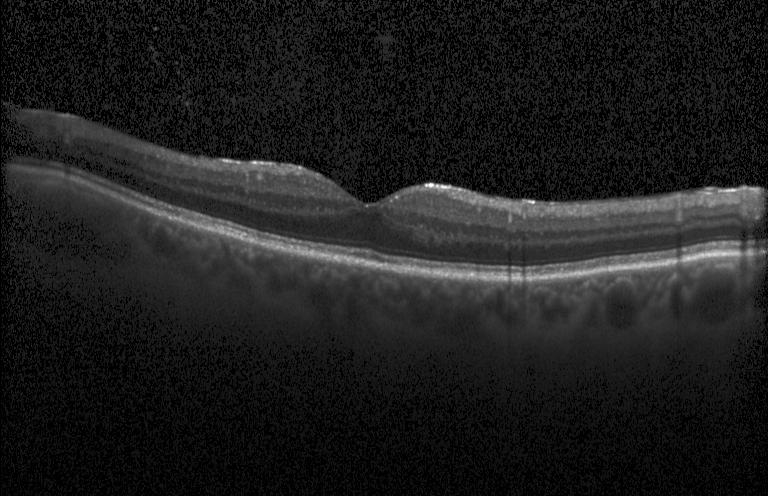 Diagnosis: no choroidal neovascularization, no diabetic macular edema, and no drusen.